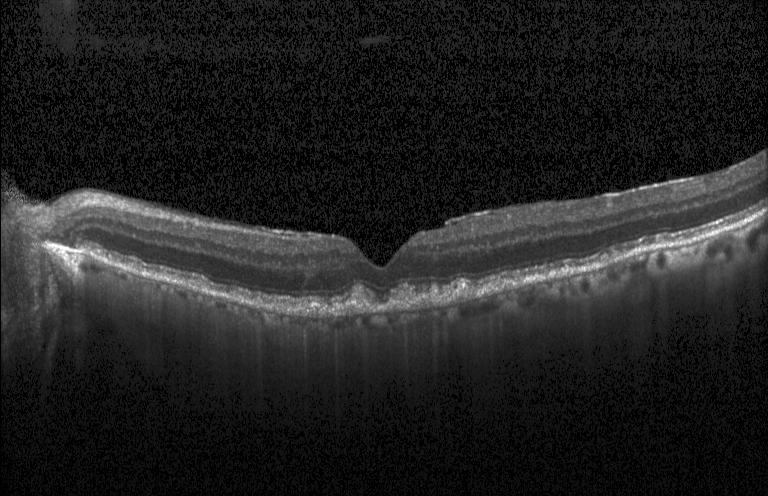
OCT B-scan showing sub-RPE drusenoid deposits.